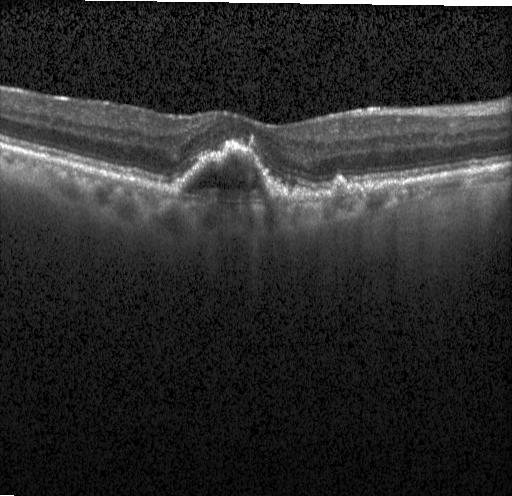
Retinal OCT B-scan. Finding: CNV.